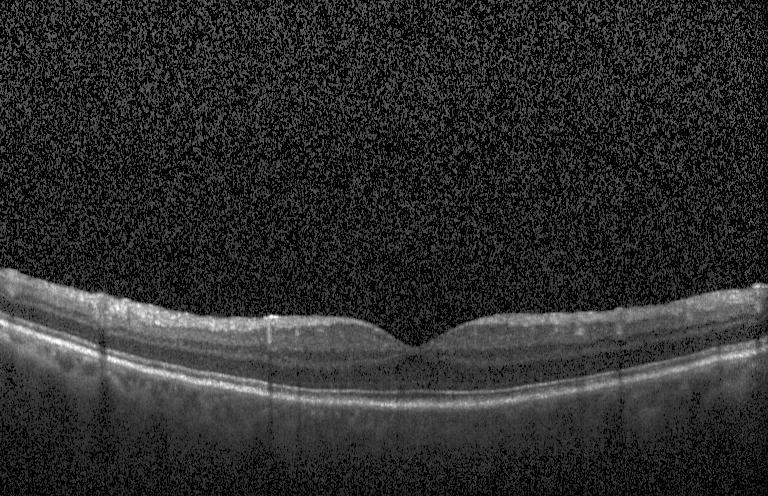
This B-scan demonstrates no choroidal neovascularization, no diabetic macular edema, and no drusen.